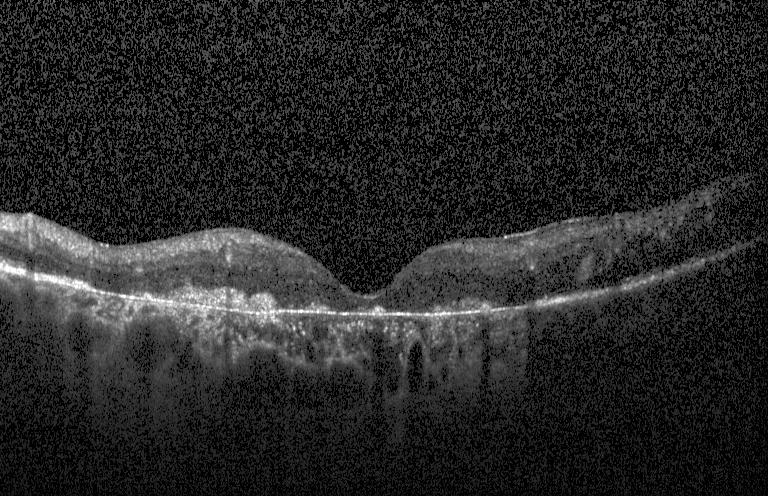
Macular scan; retinal OCT cross-section; SD-OCT; acquired on a Heidelberg Spectralis
OCT finding: choroidal neovascularization.